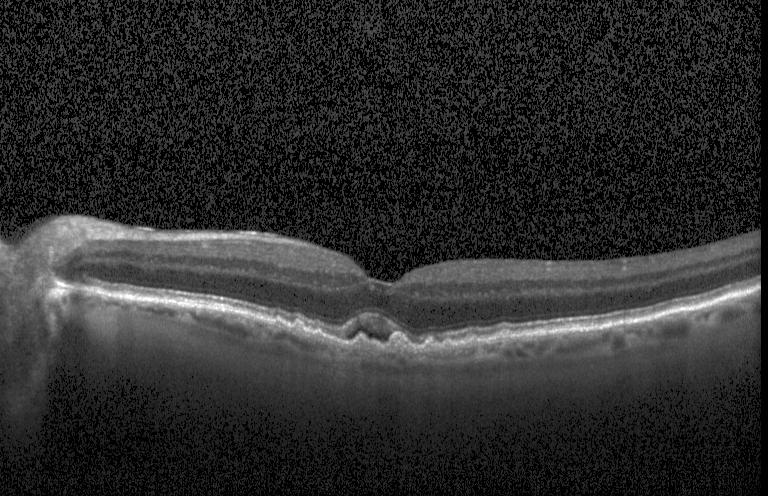

Fovea-centered · retinal OCT cross-section
Dx: a choroidal neovascular membrane.